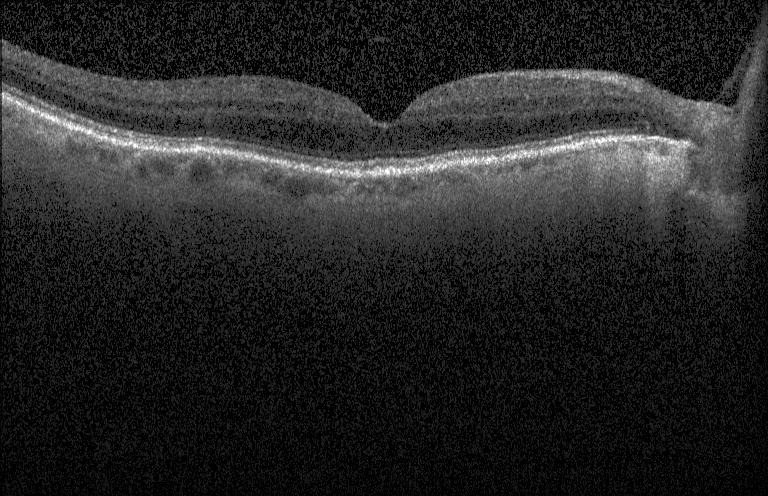
Acquired on a Heidelberg Spectralis, spectral-domain OCT, retinal OCT B-scan.
Impression: no choroidal neovascularization, no diabetic macular edema, and no drusen.